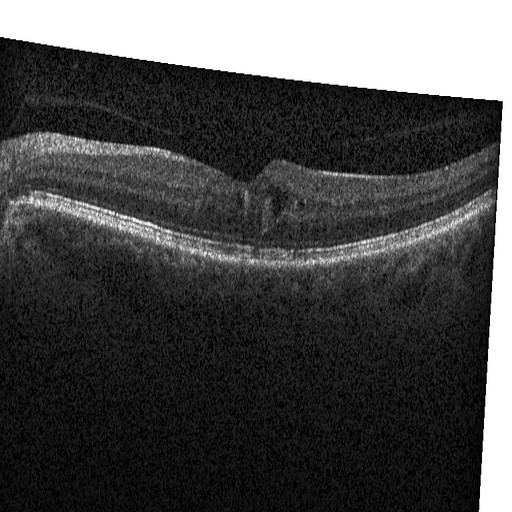 Retinal OCT cross-section, through the macula, instrument: Heidelberg Spectralis, spectral-domain OCT.
Finding: diabetic macular edema.